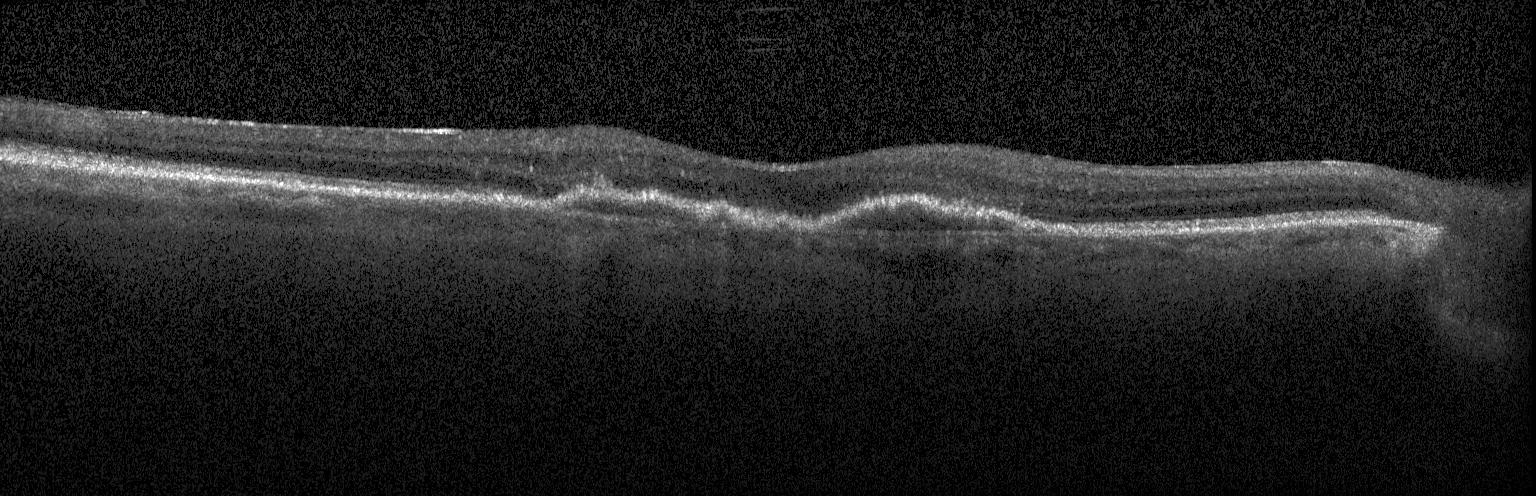

Impression: a choroidal neovascular membrane.